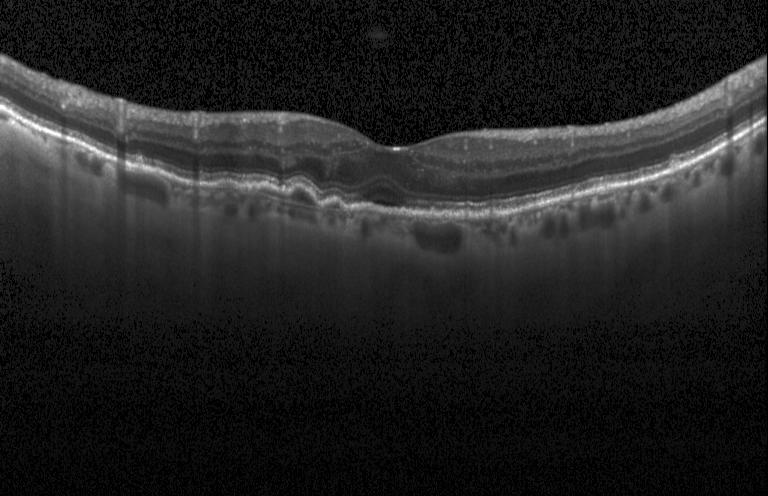

Macular scan. Instrument: Heidelberg Spectralis. Optical coherence tomography scan. Spectral-domain optical coherence tomography. Impression: CNV.